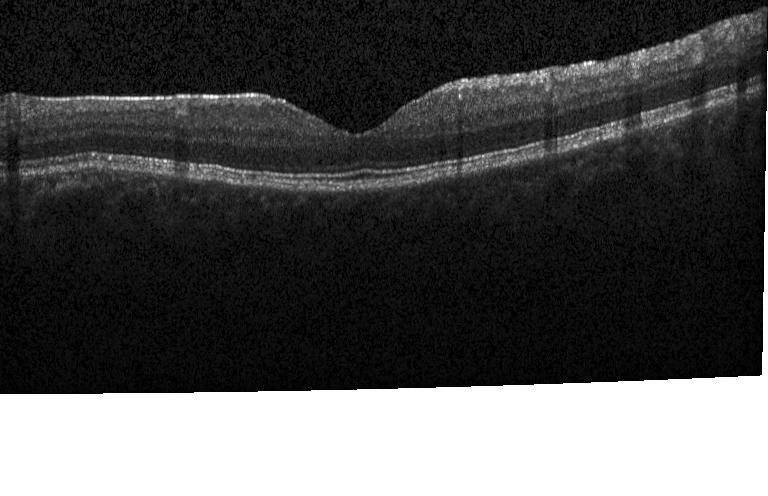
Impression: no CNV, DME, or drusen.